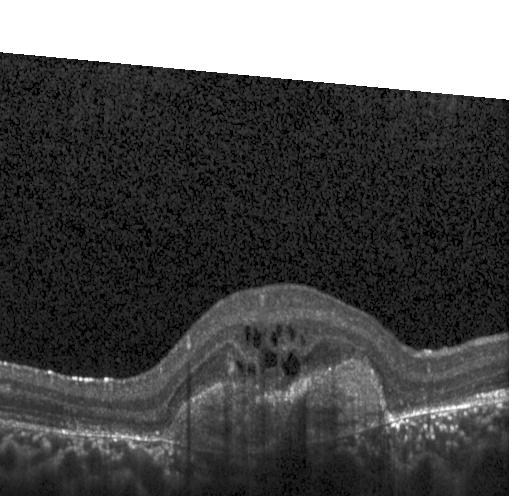
OCT scan showing CNV.